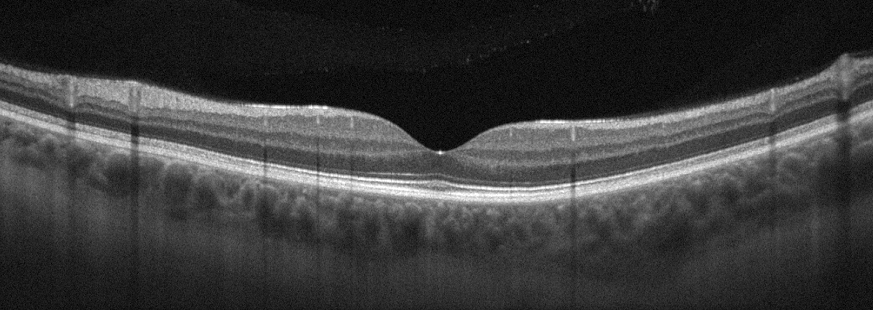 Macular OCT: absence of AMD, DME, ERM, RAO, RVO, and vitreomacular interface disease.